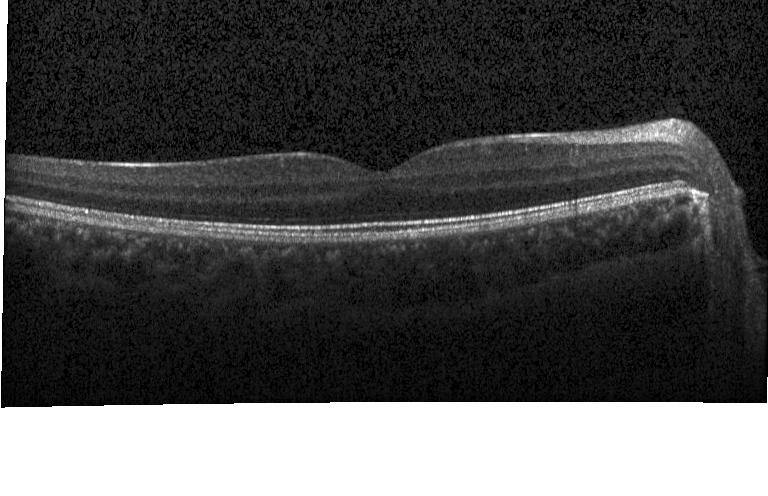 Assessment: neither CNV, DME, nor drusen.